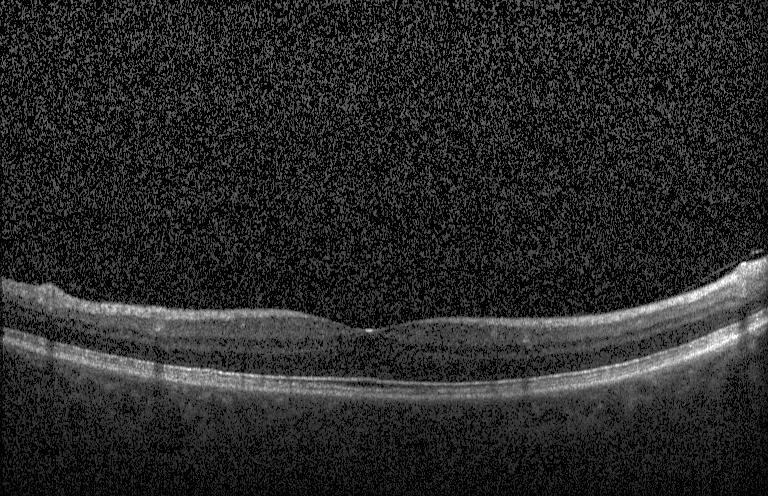
Macular scan, instrument: Heidelberg Spectralis, OCT B-scan, SD-OCT. Assessment: no CNV, no DME, and no drusen.